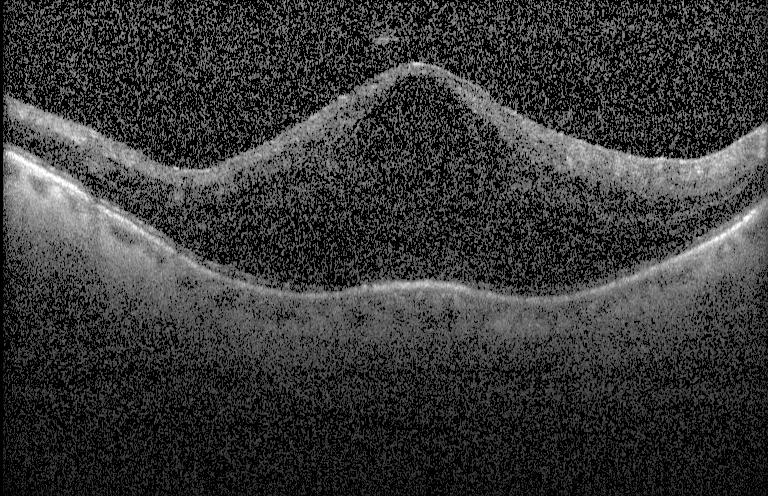

Horizontal scan through the fovea, OCT B-scan, SD-OCT — Impression: diabetic macular edema (DME).